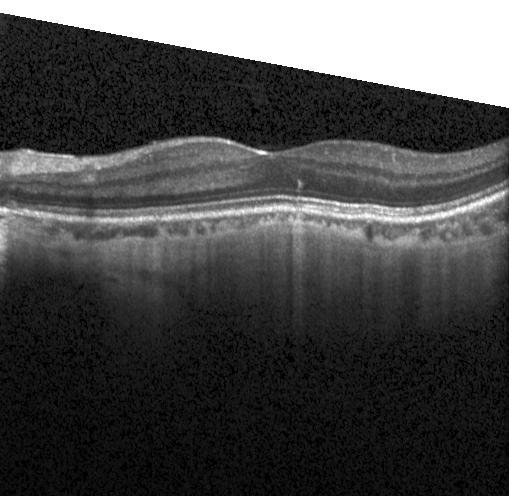
Through the macula. OCT B-scan.
This B-scan demonstrates no choroidal neovascularization, diabetic macular edema, or drusen.